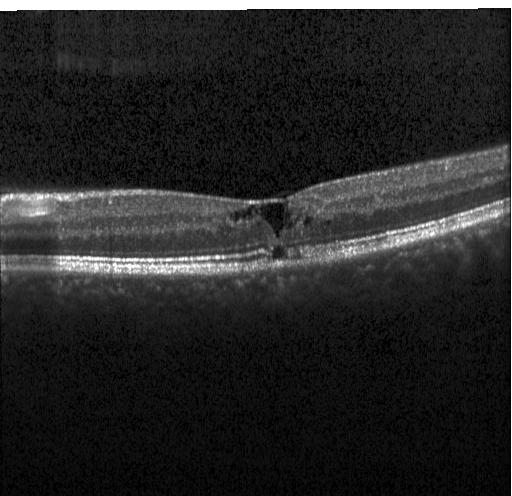 Diagnosis: diabetic macular edema (DME).